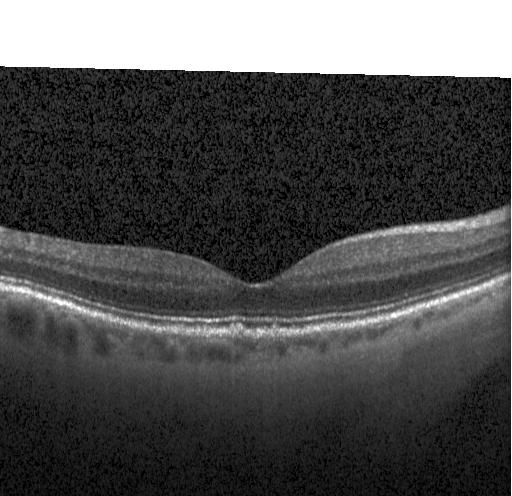
Spectral-domain OCT · OCT B-scan · acquired on a Heidelberg Spectralis — Diagnosis: drusen.